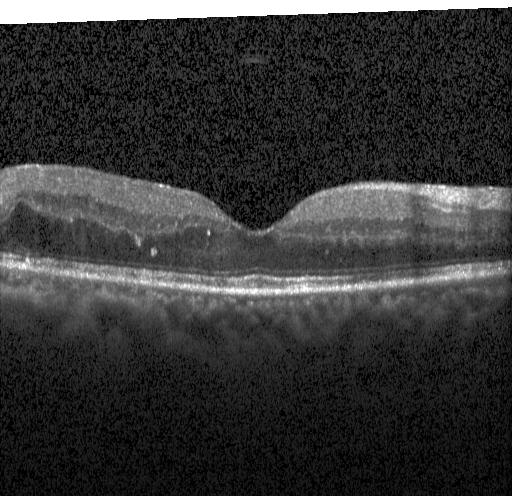
Optical coherence tomography B-scan — Diagnosis: DME.